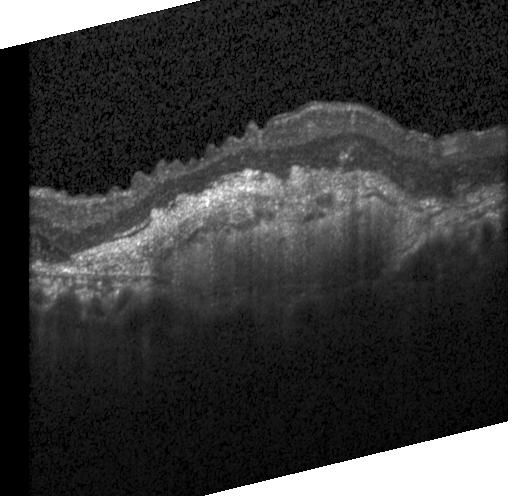
Diagnosis: CNV.